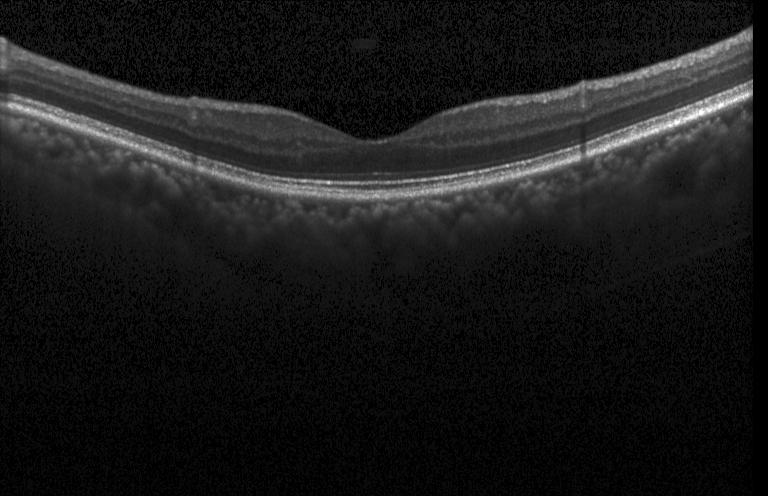

OCT B-scan, SD-OCT, fovea-centered
The scan shows no choroidal neovascularization, diabetic macular edema, or drusen.